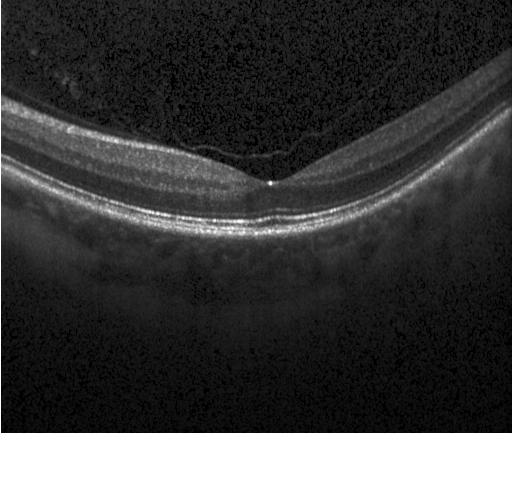

OCT line scan, fovea-centered. Impression: neither choroidal neovascularization, diabetic macular edema, nor drusen.